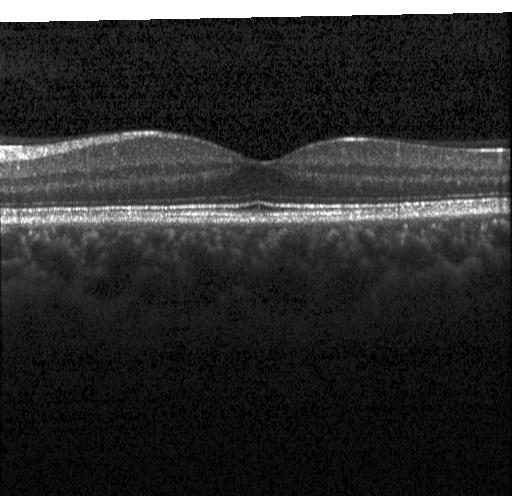

OCT scan showing no choroidal neovascularization, no diabetic macular edema, and no drusen.